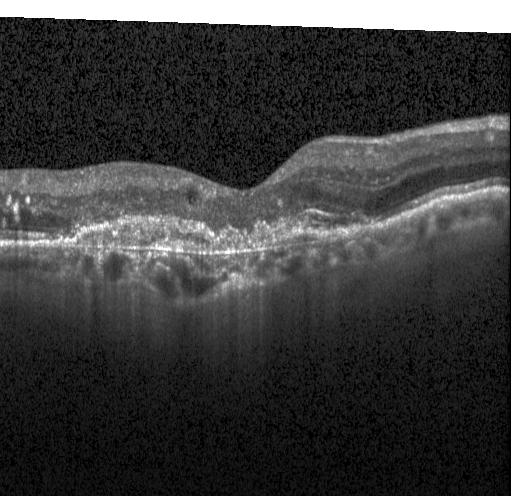

Optical coherence tomography B-scan · through the macula · SD-OCT. Impression: a choroidal neovascular membrane.